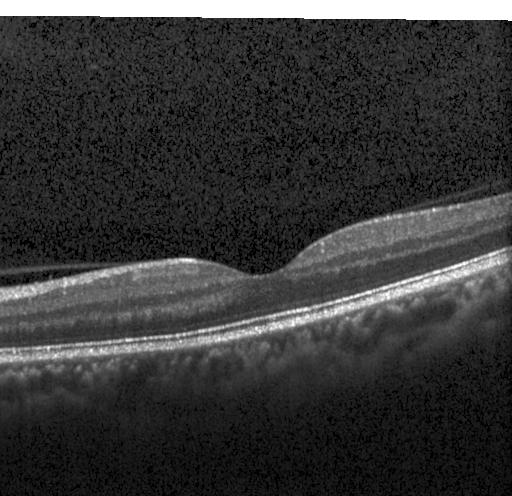

Impression: no evidence of CNV, DME, or drusen.